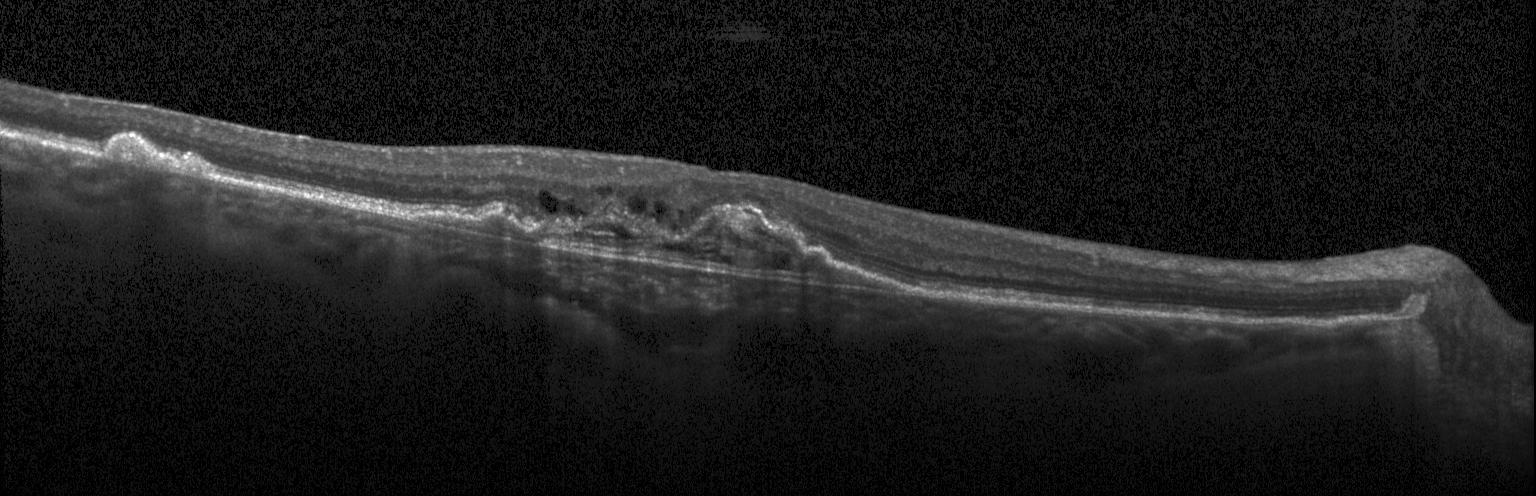 Retinal OCT cross-section, instrument: Heidelberg Spectralis
Finding: a choroidal neovascular membrane.